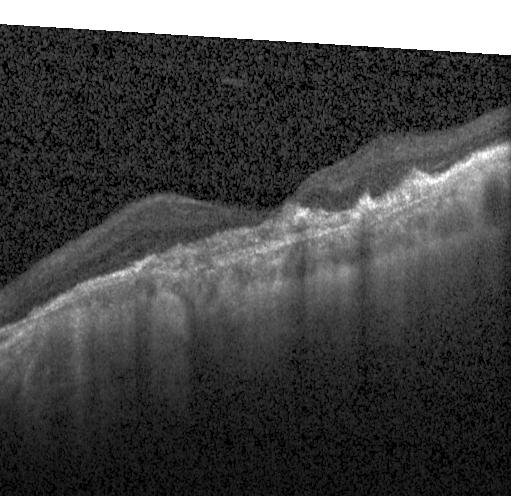

OCT B-scan — This B-scan demonstrates a choroidal neovascular membrane.